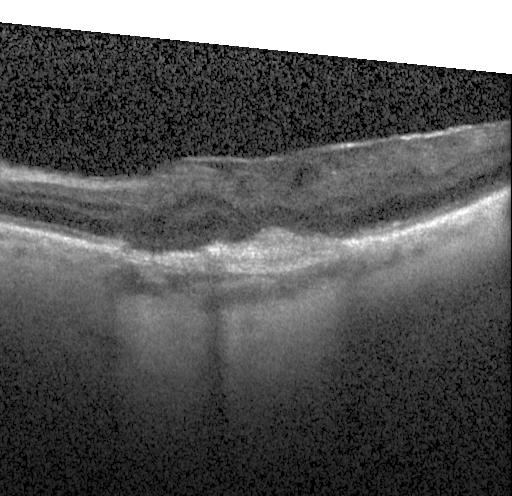 OCT B-scan. Instrument: Heidelberg Spectralis. Spectral-domain optical coherence tomography. Centered on the fovea
Macular OCT: a choroidal neovascular membrane.